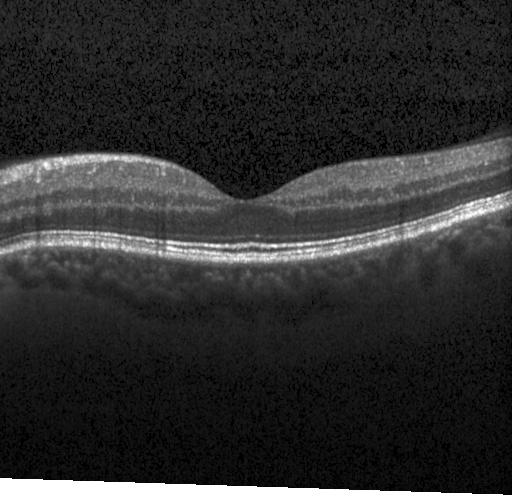 Macular scan, spectral-domain optical coherence tomography, optical coherence tomography scan, Heidelberg Spectralis OCT system
Diagnosis: no evidence of choroidal neovascularization, diabetic macular edema, or drusen.